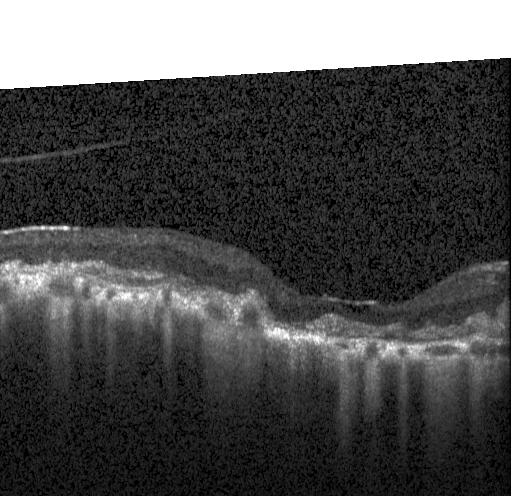

Impression: choroidal neovascularization (CNV).